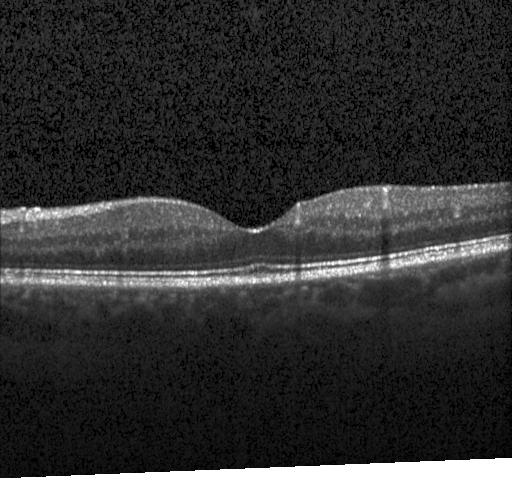
Assessment: no choroidal neovascularization, diabetic macular edema, or drusen.